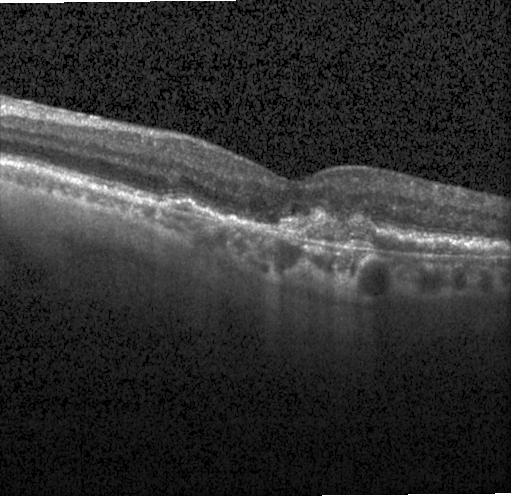
Heidelberg Spectralis; spectral-domain OCT; OCT line scan. Diagnosis: CNV.